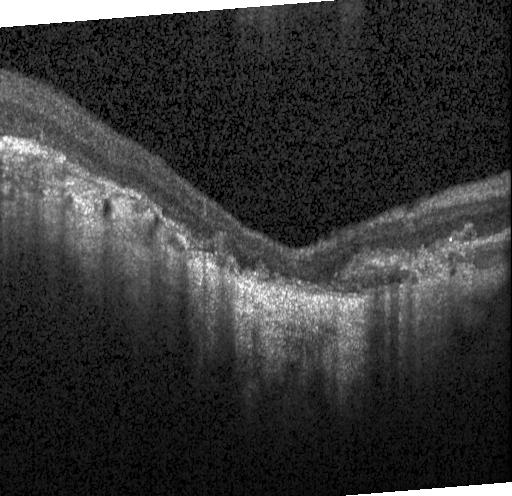 Optical coherence tomography scan; spectral-domain OCT — This B-scan demonstrates a choroidal neovascular membrane.